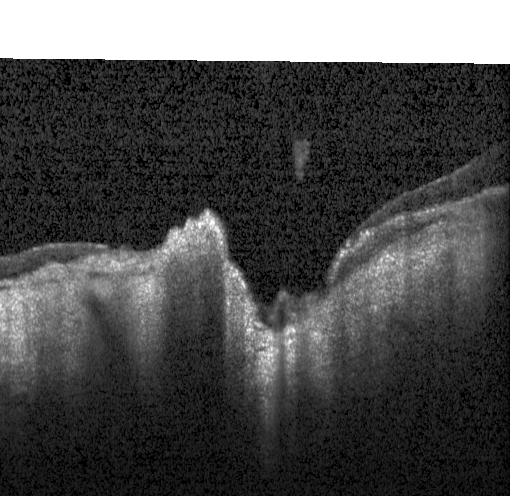 Diagnosis: a choroidal neovascular membrane.